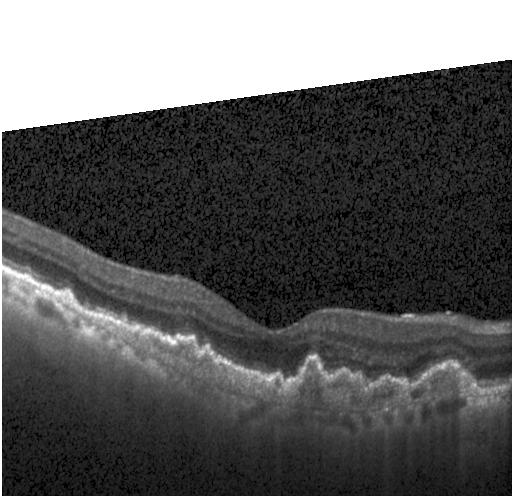
SD-OCT, macular scan, OCT B-scan. OCT finding: a choroidal neovascular membrane.